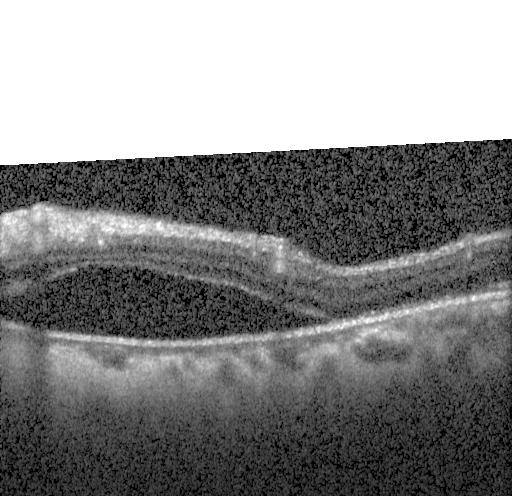 Retinal OCT cross-section showing a choroidal neovascular membrane.